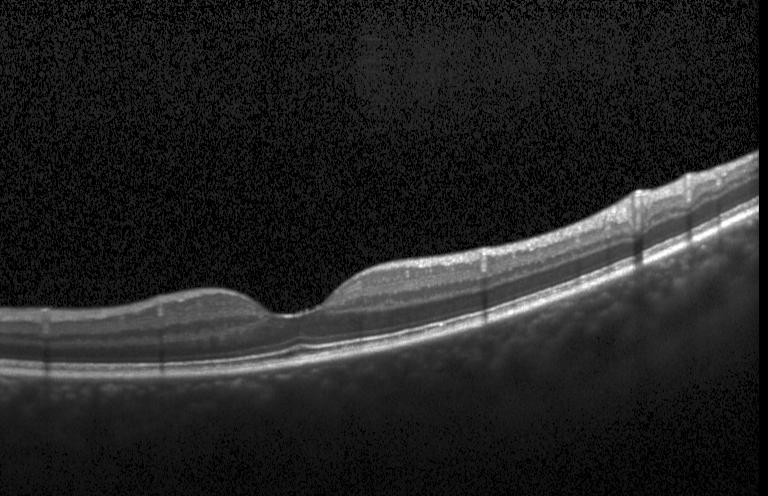 Acquired on a Heidelberg Spectralis; SD-OCT; optical coherence tomography B-scan
The scan shows no evidence of choroidal neovascularization, diabetic macular edema, or drusen.